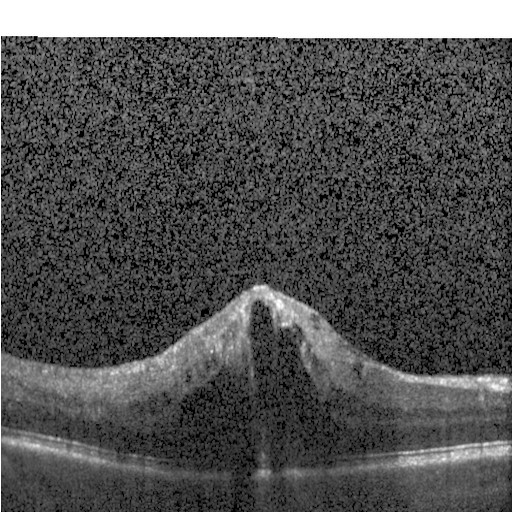 Impression: DME.